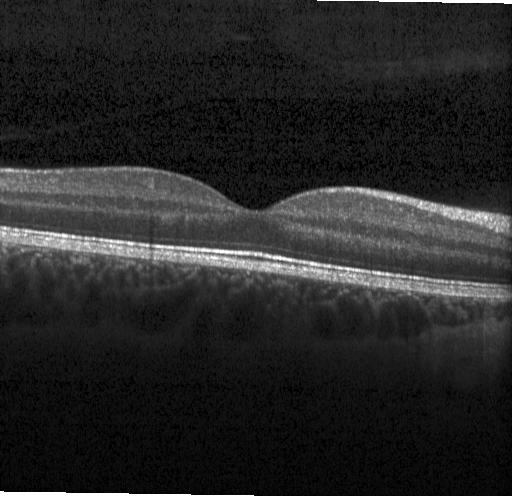 Diagnosis: no choroidal neovascularization, no diabetic macular edema, and no drusen.